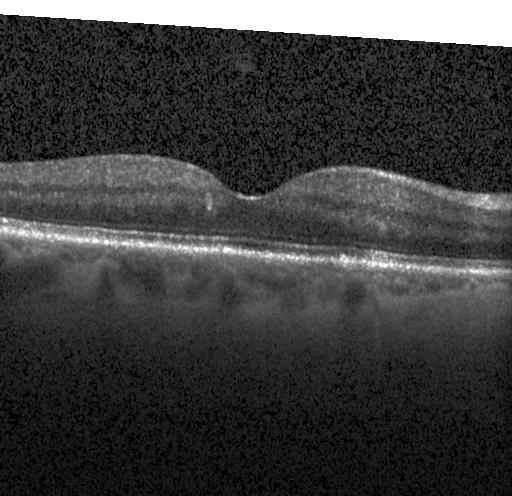

SD-OCT. Optical coherence tomography B-scan. Instrument: Heidelberg Spectralis. Horizontal scan through the fovea — Diagnosis: no choroidal neovascularization, diabetic macular edema, or drusen.